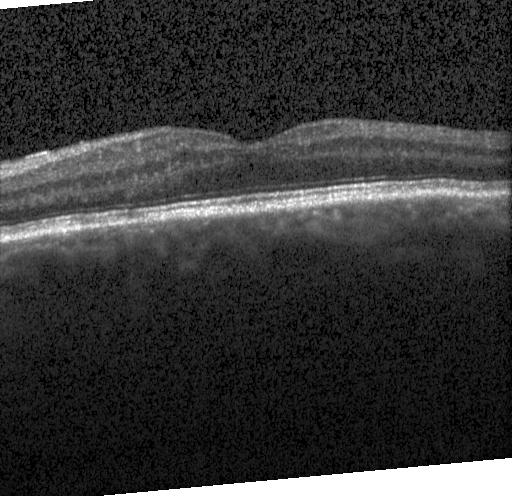

Heidelberg Spectralis OCT system, OCT B-scan. Impression: neither CNV, DME, nor drusen.